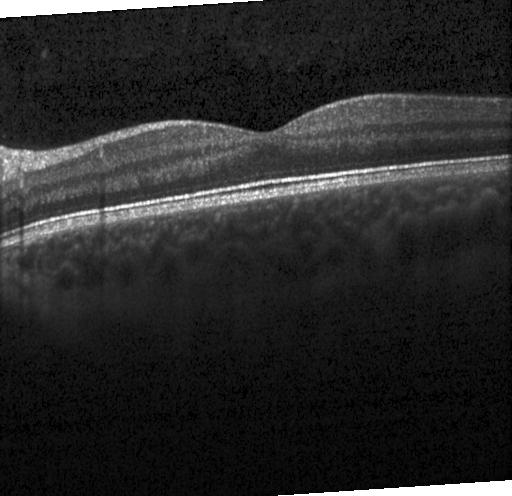 Instrument: Heidelberg Spectralis, horizontal scan through the fovea, SD-OCT, OCT line scan — This B-scan demonstrates no CNV, DME, or drusen.